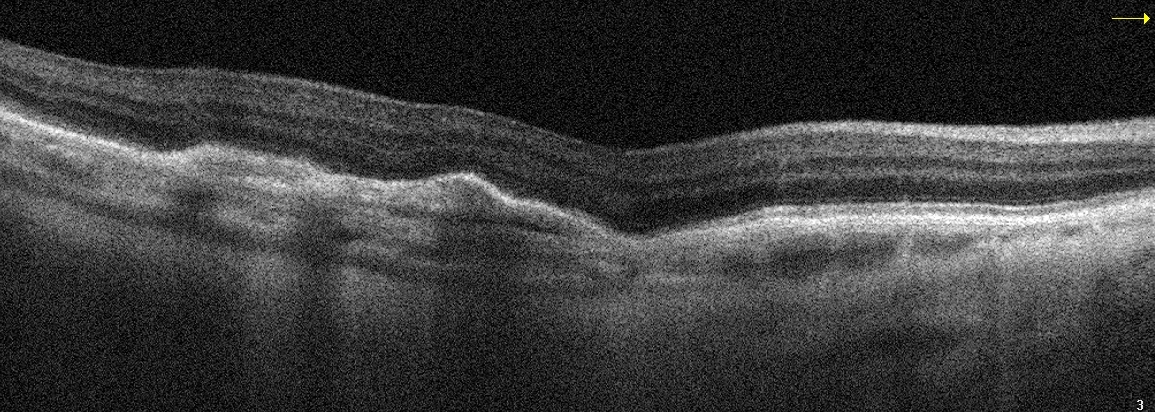
Macular OCT: age-related macular degeneration.